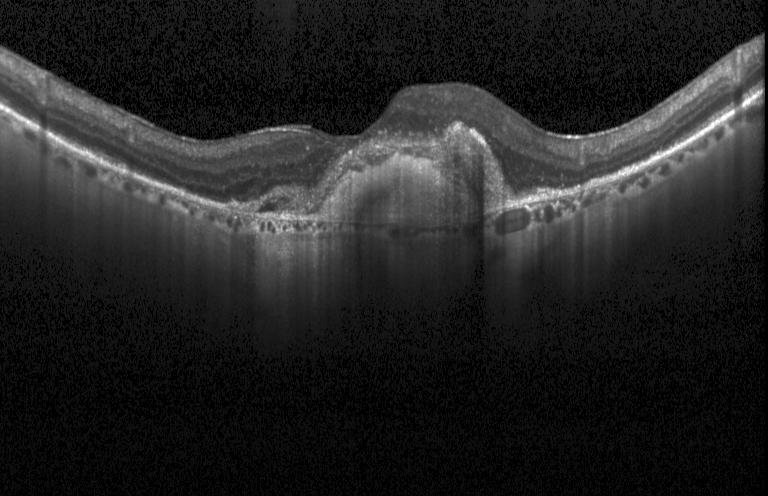
Retinal OCT B-scan; SD-OCT; Heidelberg Spectralis OCT system
This B-scan demonstrates choroidal neovascularization (CNV).